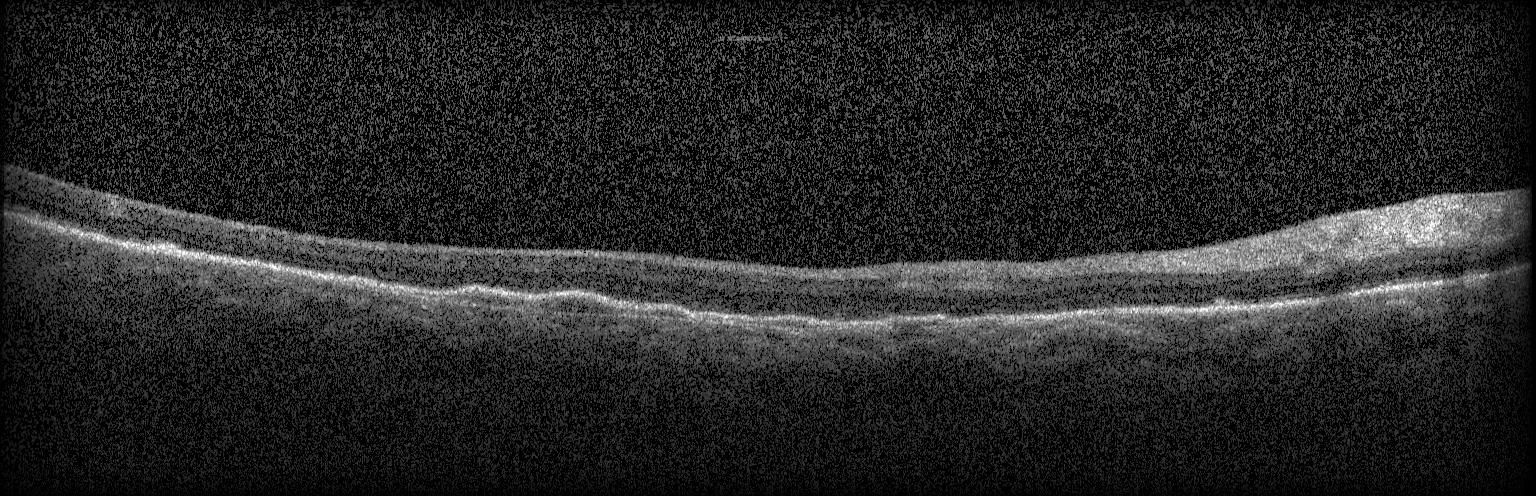
Retinal OCT cross-section showing CNV.